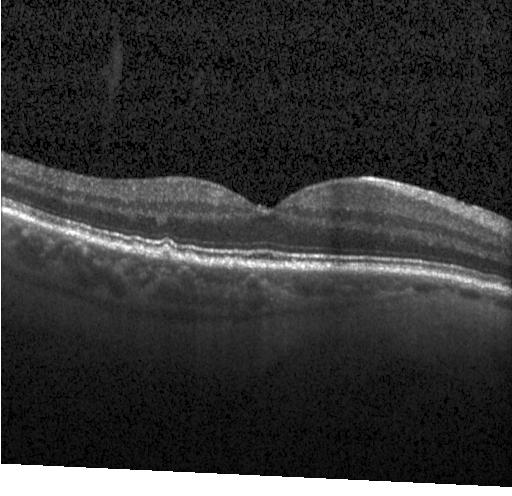 Optical coherence tomography B-scan
This B-scan demonstrates multiple drusen.